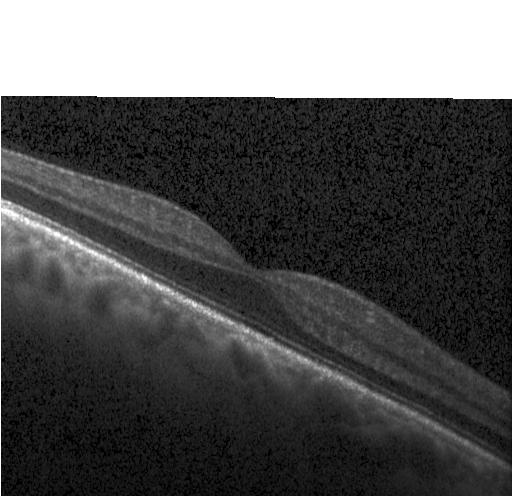
Retinal OCT B-scan, instrument: Heidelberg Spectralis, fovea-centered, spectral-domain optical coherence tomography.
The scan shows no choroidal neovascularization, diabetic macular edema, or drusen.